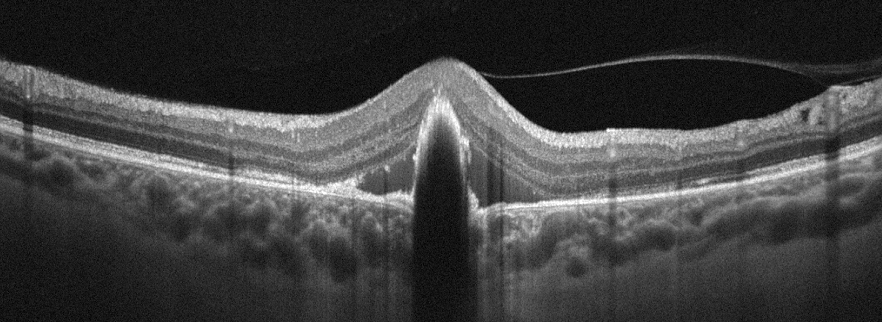 OCT line scan, left eye. Impression: AMD.